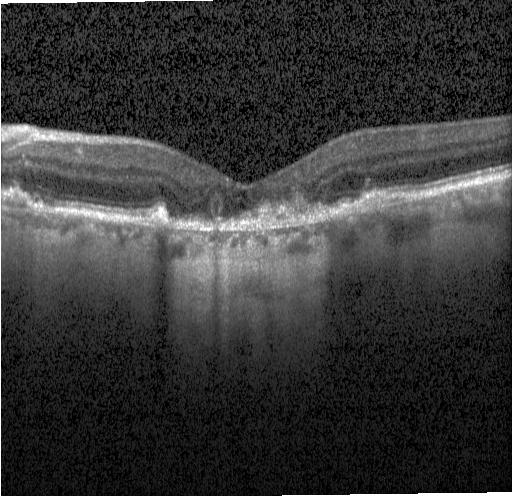

OCT scan showing choroidal neovascularization.